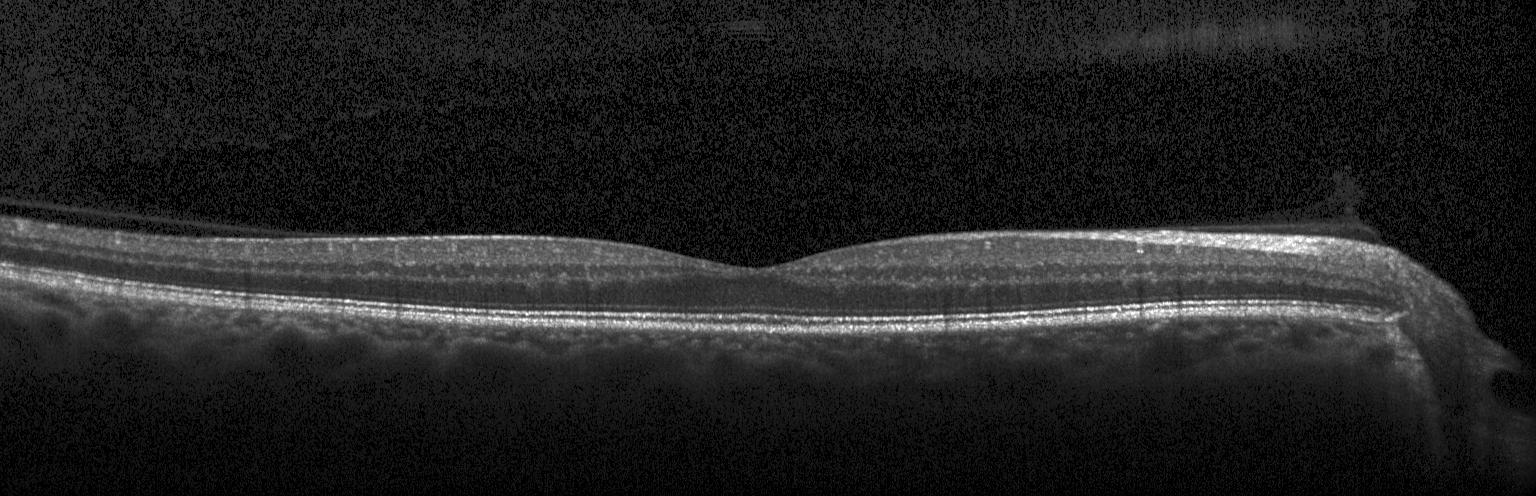
Dx: no CNV, DME, or drusen.